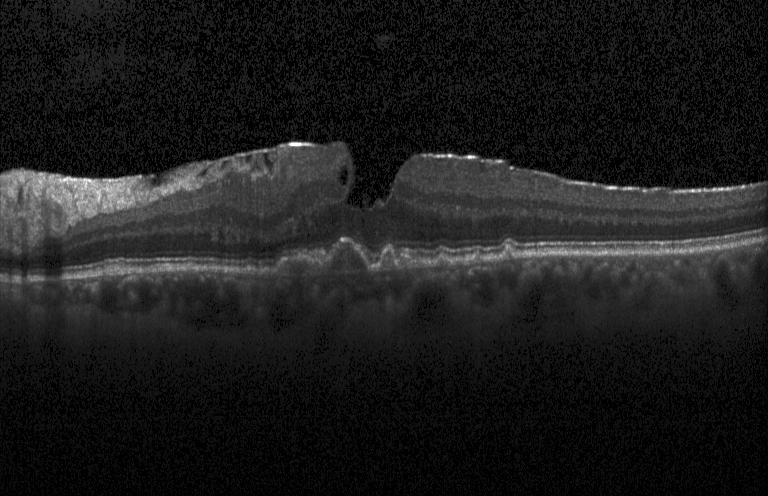 Diagnosis: choroidal neovascularization (CNV).